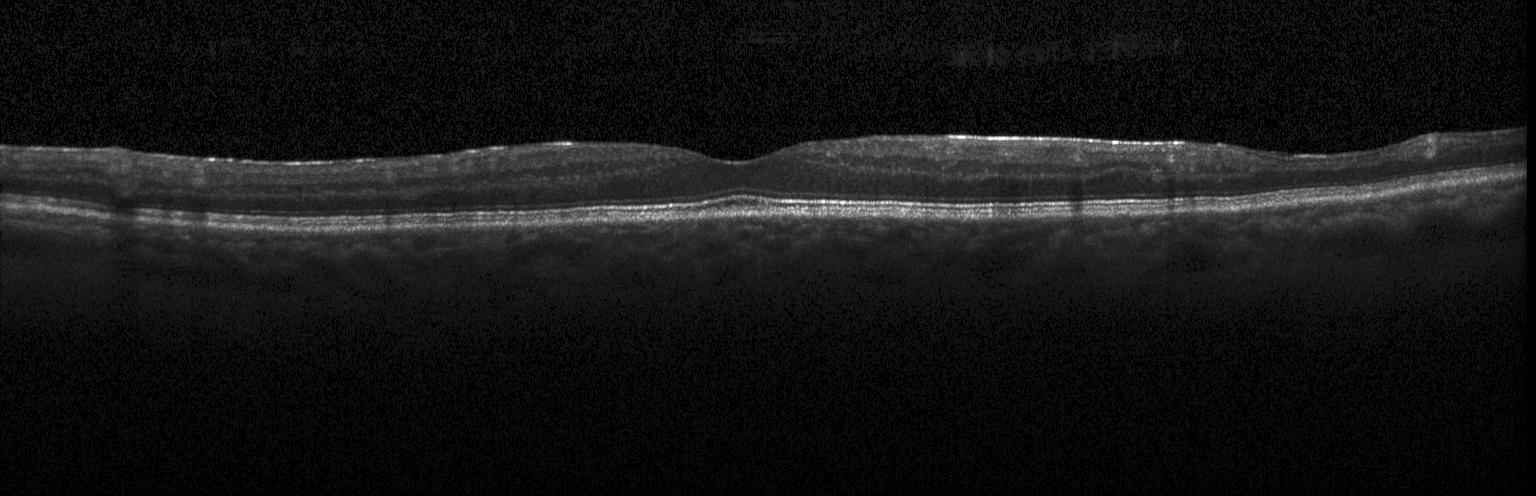

Heidelberg Spectralis. OCT line scan — Diagnosis: neither choroidal neovascularization, diabetic macular edema, nor drusen.